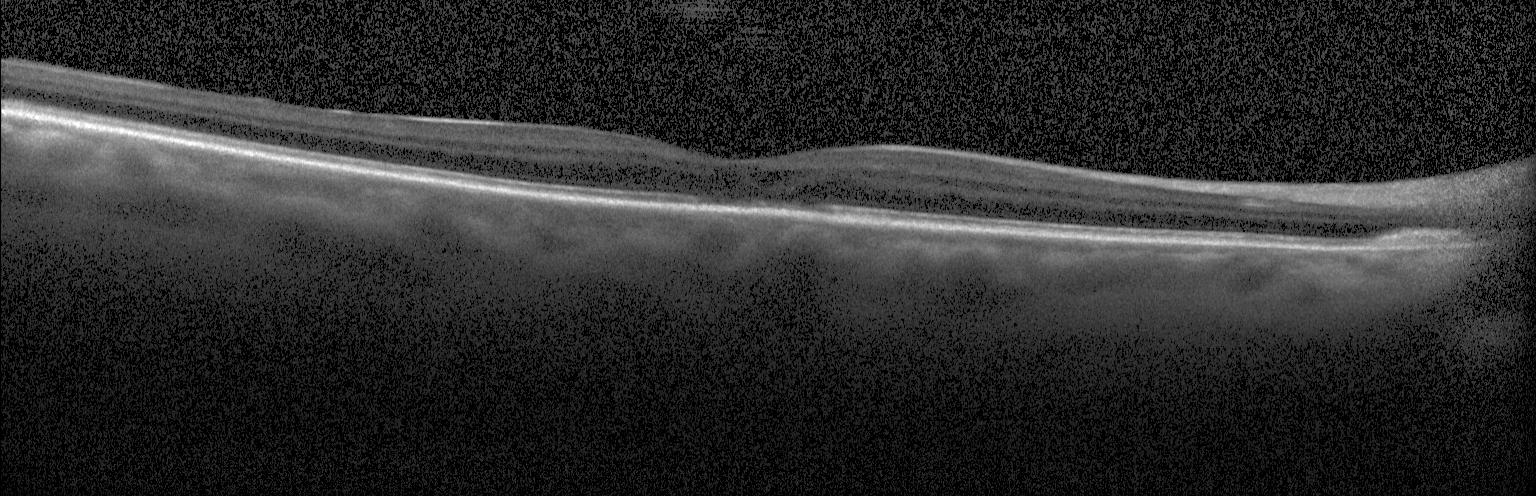 Macular OCT: diabetic macular edema (DME).